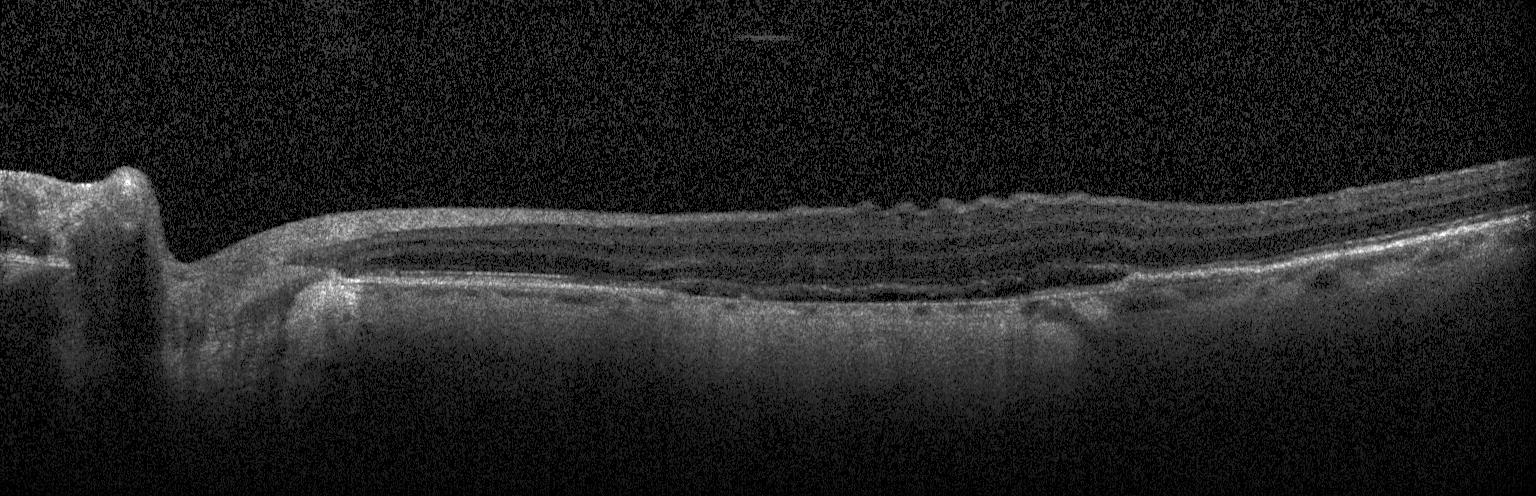 OCT finding: CNV.